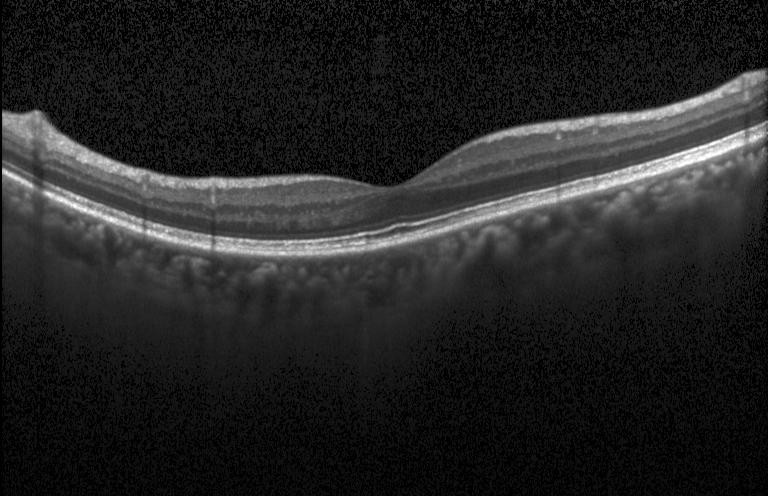

OCT B-scan — Finding: neither choroidal neovascularization, diabetic macular edema, nor drusen.